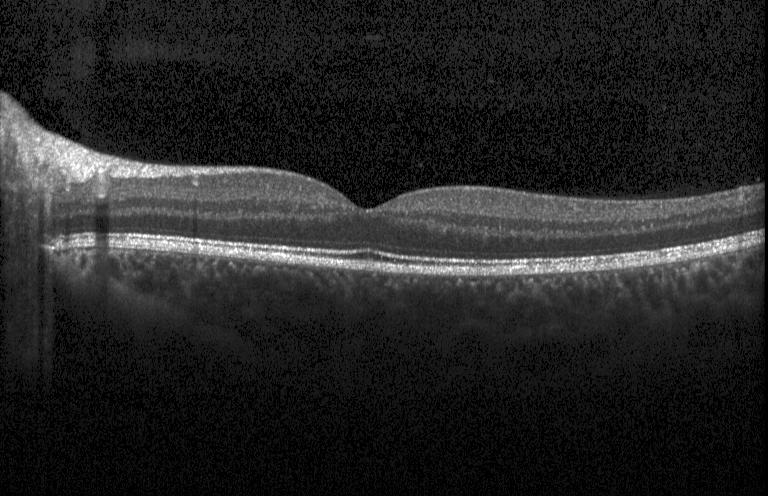 Spectral-domain optical coherence tomography. Centered on the fovea. Instrument: Heidelberg Spectralis. OCT line scan
Macular OCT: neither choroidal neovascularization, diabetic macular edema, nor drusen.